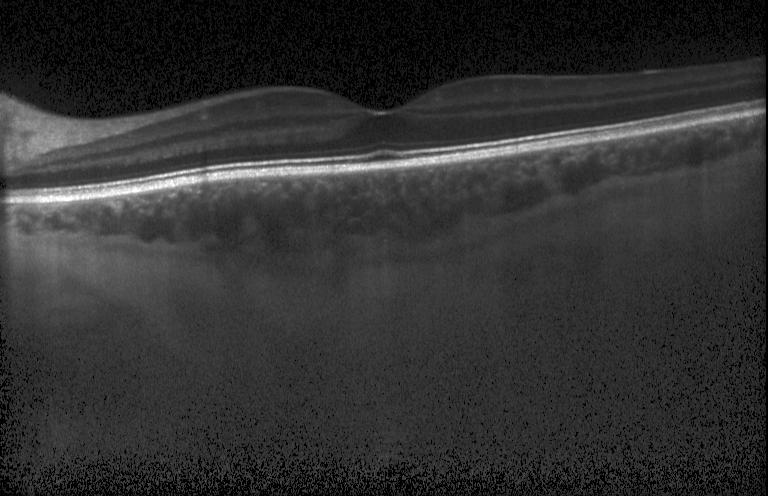
Impression: no CNV, no DME, and no drusen.